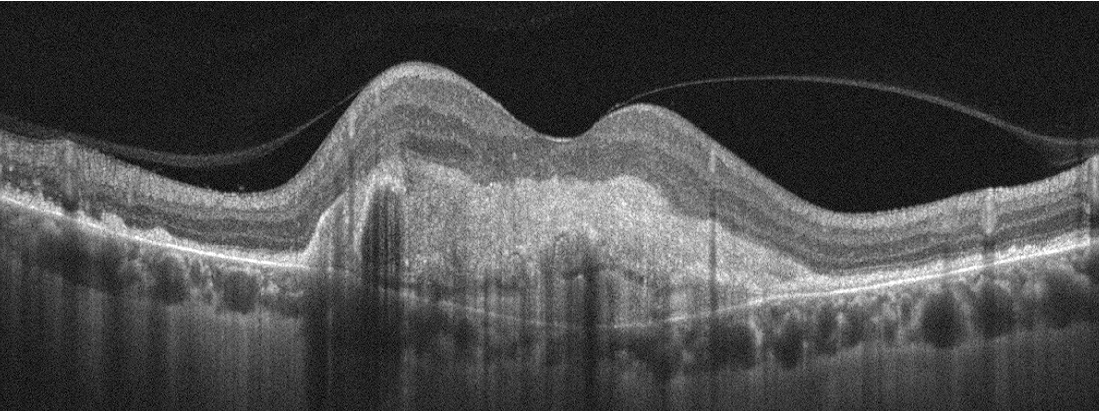 Retinal OCT B-scan.
Diagnosis: age-related macular degeneration (AMD).